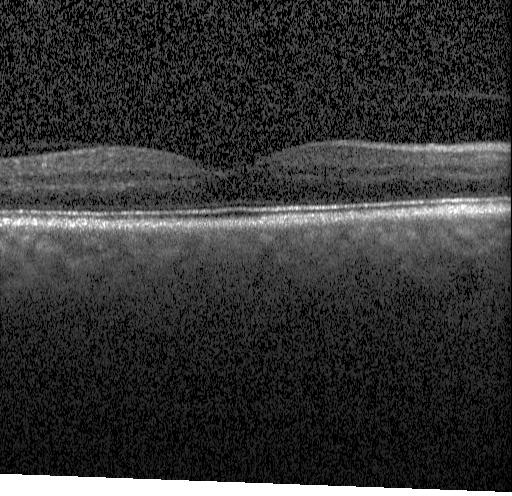
OCT B-scan · Heidelberg Spectralis OCT system · macular scan.
OCT finding: neither choroidal neovascularization, diabetic macular edema, nor drusen.